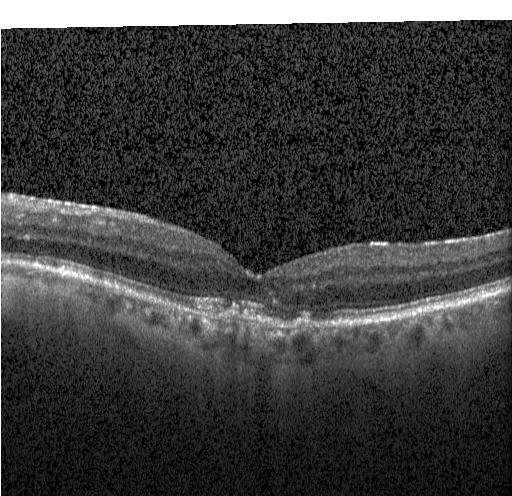

OCT line scan. Heidelberg Spectralis OCT system. Spectral-domain OCT
Finding: CNV.